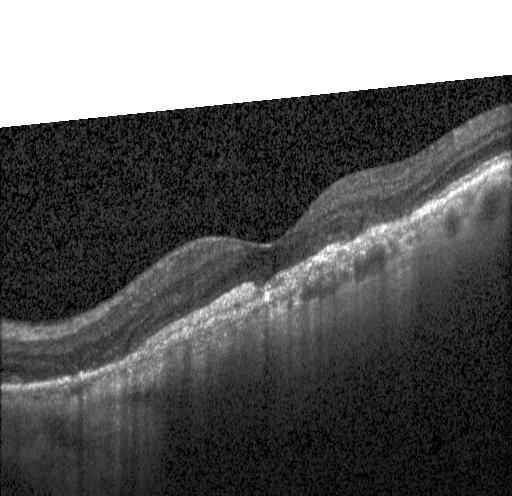 OCT finding: a choroidal neovascular membrane.